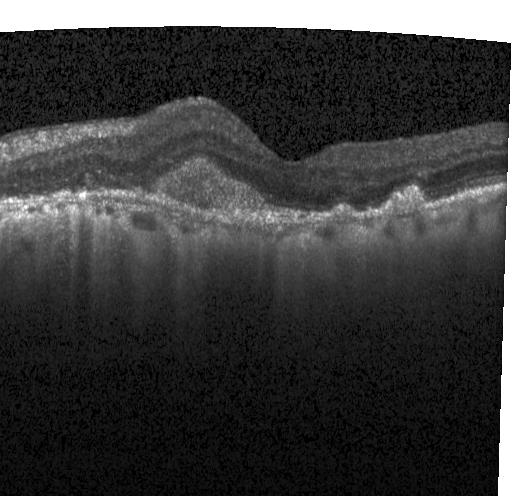

Optical coherence tomography scan; spectral-domain optical coherence tomography; Heidelberg Spectralis; fovea-centered
Dx: a choroidal neovascular membrane.